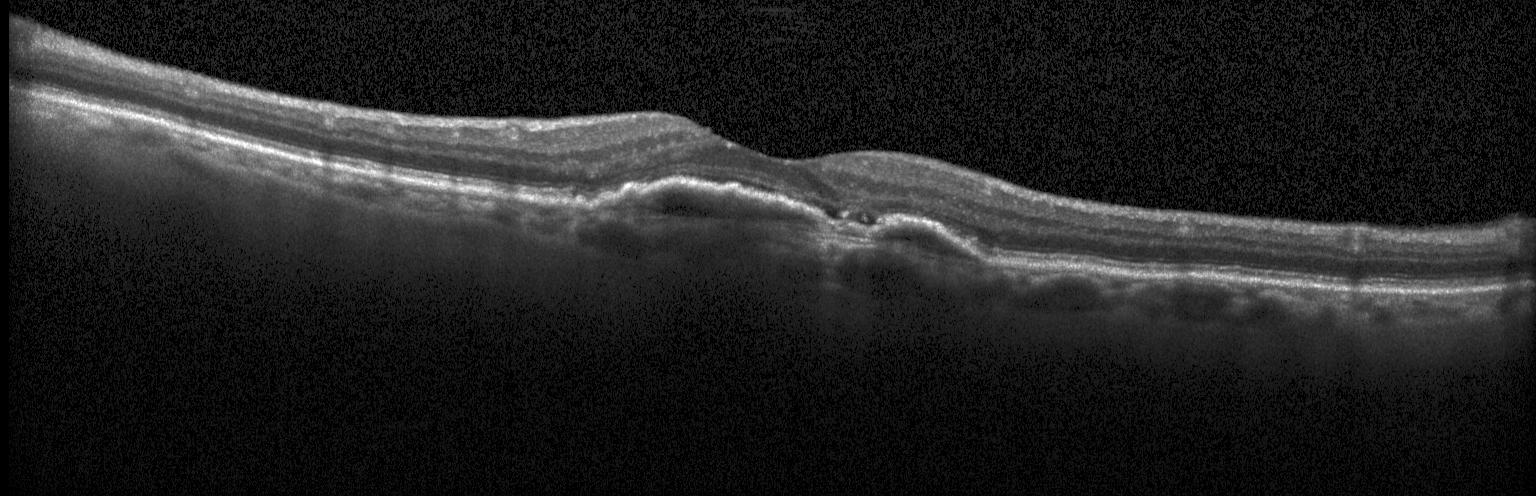

Optical coherence tomography scan, instrument: Heidelberg Spectralis
Finding: a choroidal neovascular membrane.